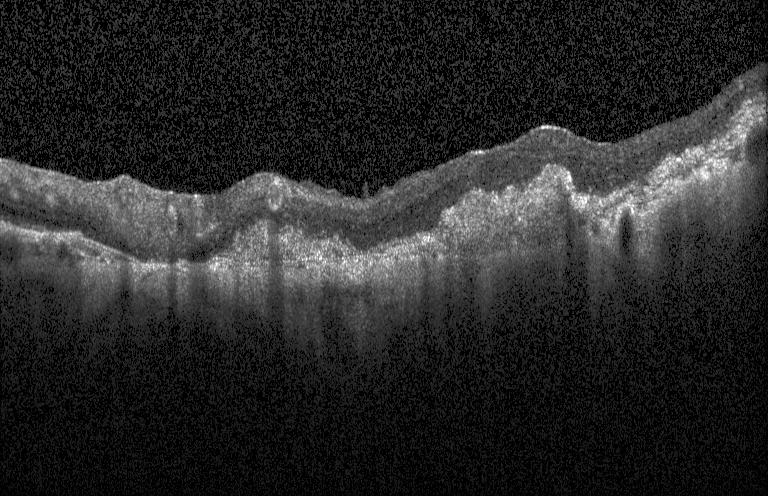
Spectral-domain OCT B-scan: choroidal neovascularization.